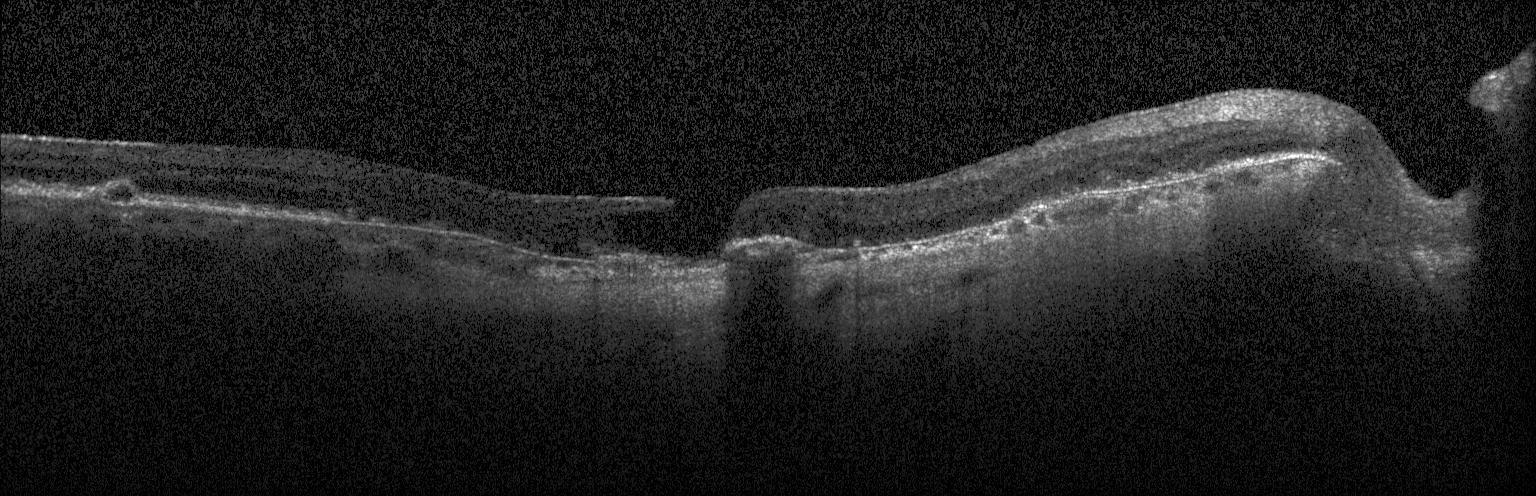
Retinal OCT cross-section showing a choroidal neovascular membrane.